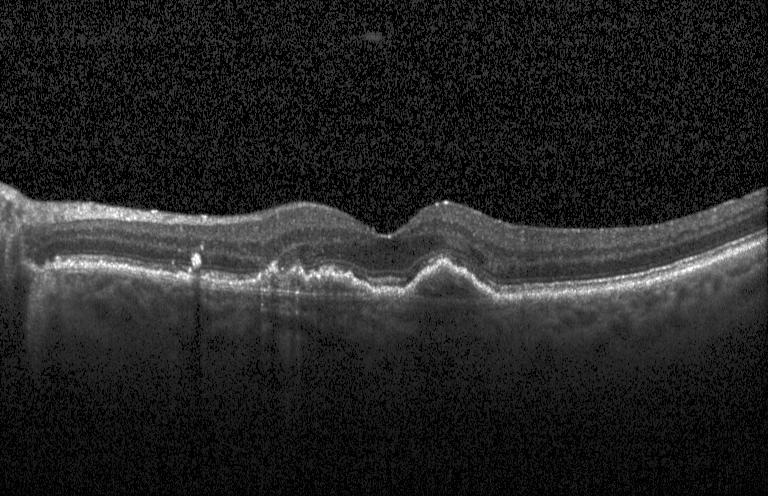

SD-OCT. Optical coherence tomography scan. Diagnosis: choroidal neovascularization.